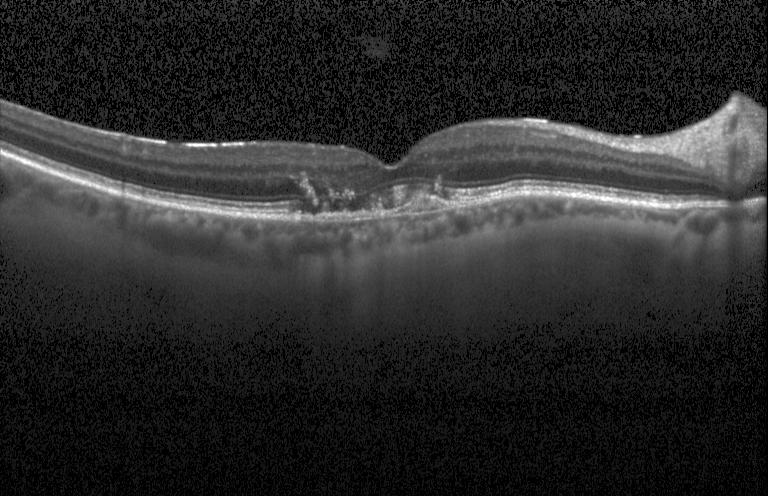 Through the macula; optical coherence tomography scan; instrument: Heidelberg Spectralis; spectral-domain optical coherence tomography.
OCT finding: a choroidal neovascular membrane.